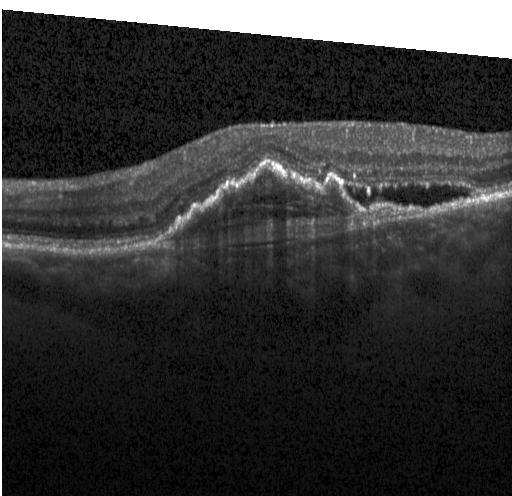

Optical coherence tomography B-scan, acquired on a Heidelberg Spectralis.
This B-scan demonstrates CNV.